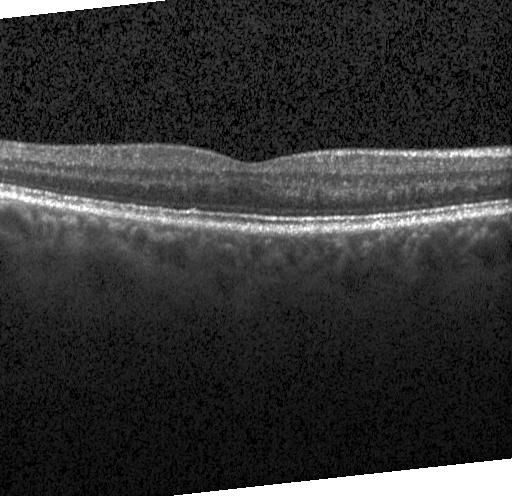
Macular scan, spectral-domain optical coherence tomography, retinal OCT B-scan, Heidelberg Spectralis. Impression: no choroidal neovascularization, no diabetic macular edema, and no drusen.